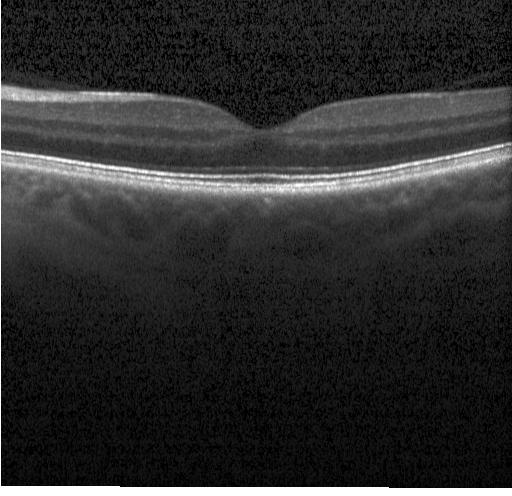 No CNV, DME, or drusen.